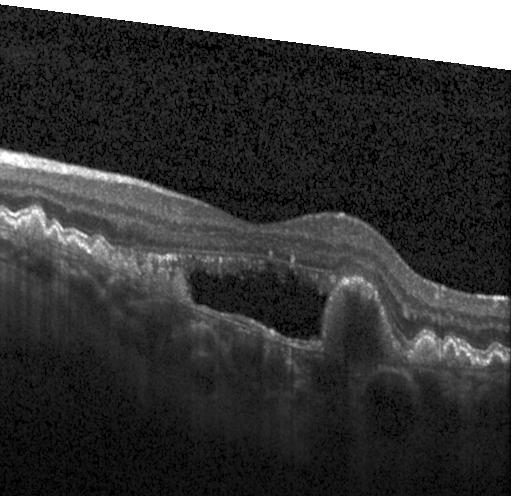

Spectral-domain optical coherence tomography, optical coherence tomography B-scan, acquired on a Heidelberg Spectralis.
Assessment: a choroidal neovascular membrane.